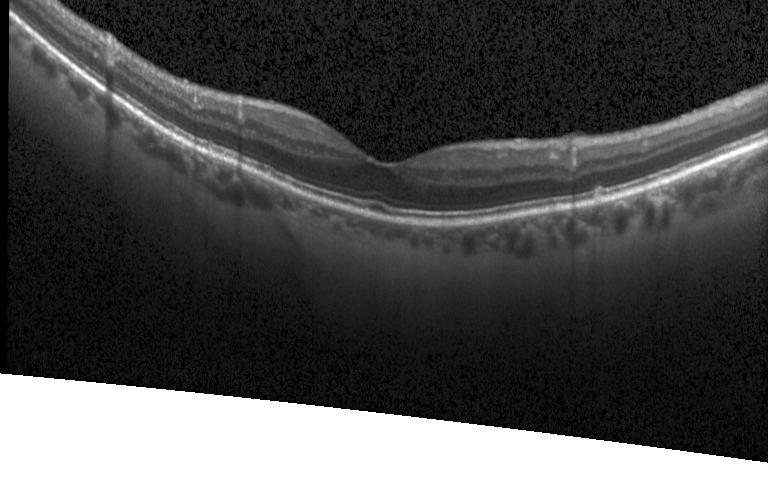

Macular OCT demonstrating sub-RPE drusenoid deposits.